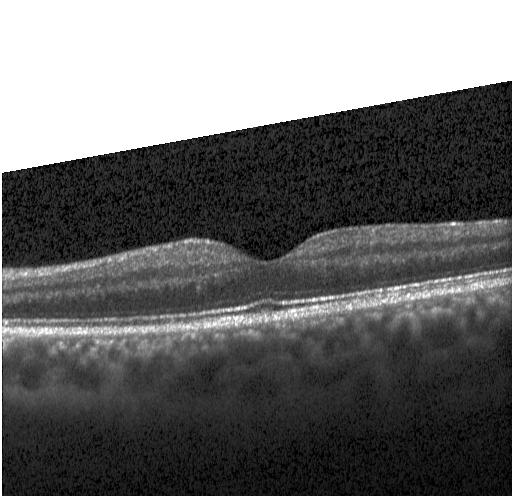 Macular scan, spectral-domain OCT, retinal OCT B-scan
Finding: no CNV, DME, or drusen.